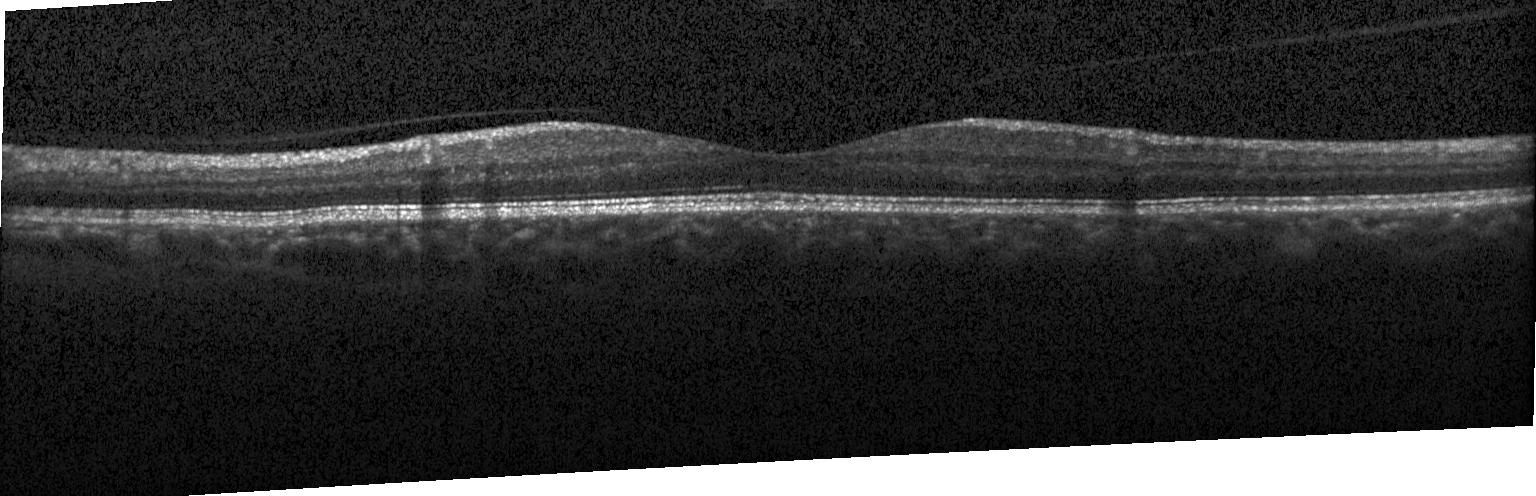 Heidelberg Spectralis OCT system · optical coherence tomography B-scan · spectral-domain optical coherence tomography. Assessment: neither CNV, DME, nor drusen.